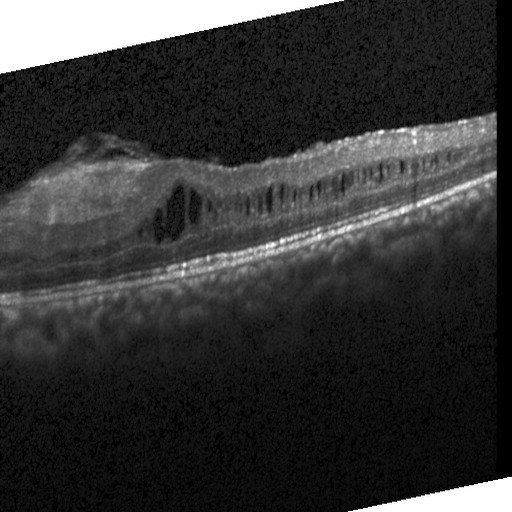
Optical coherence tomography B-scan.
Finding: diabetic macular edema (DME).